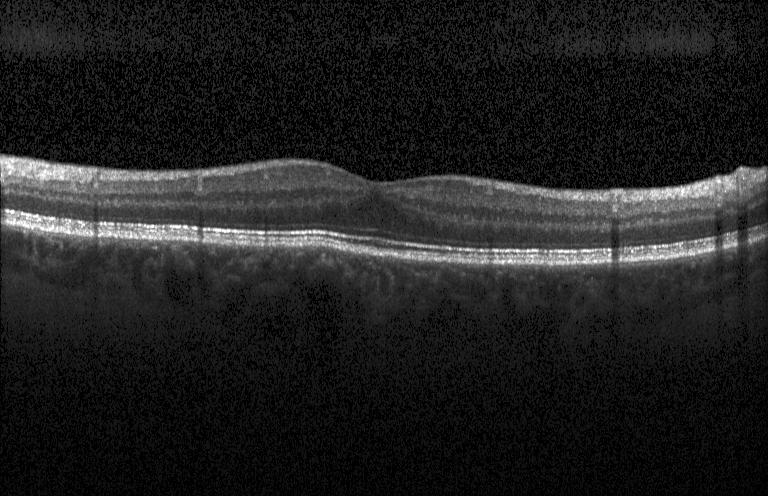 Finding: no choroidal neovascularization, diabetic macular edema, or drusen.